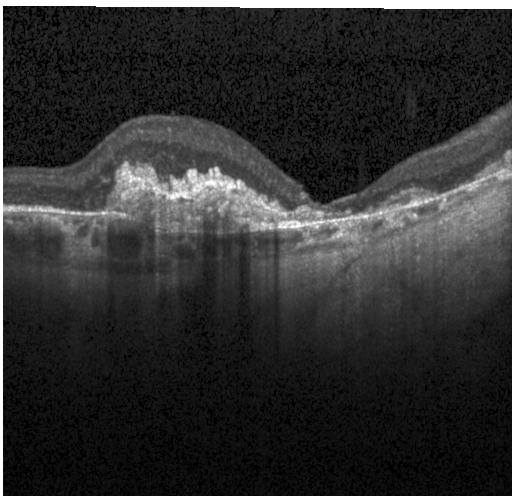
This B-scan demonstrates a choroidal neovascular membrane.